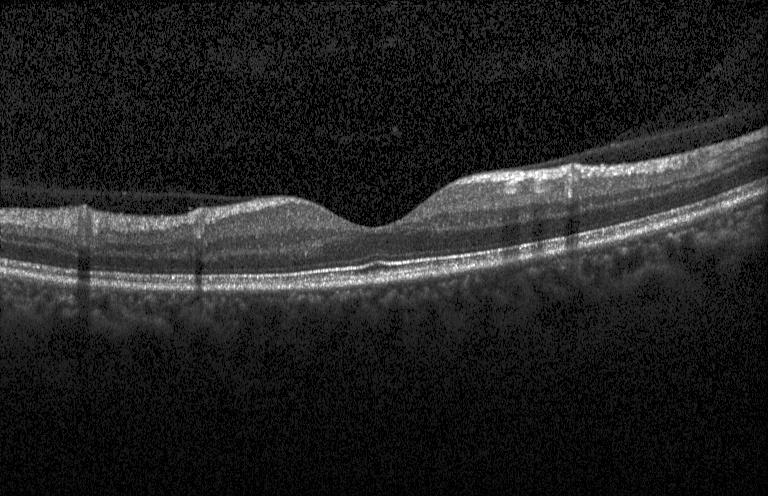 Assessment: neither choroidal neovascularization, diabetic macular edema, nor drusen.